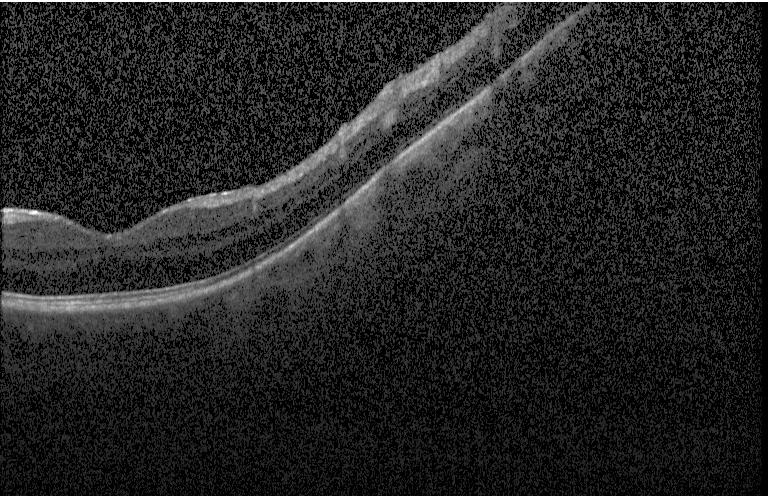 Heidelberg Spectralis OCT system; retinal OCT cross-section — No choroidal neovascularization, diabetic macular edema, or drusen.